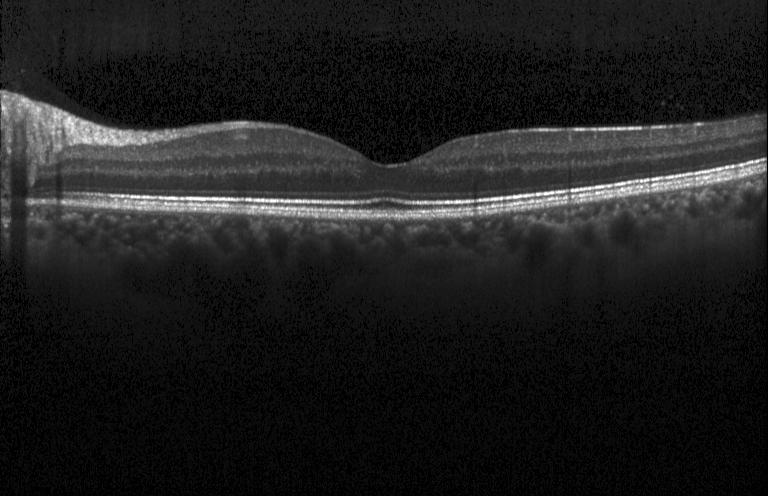 SD-OCT, OCT line scan. Diagnosis: no choroidal neovascularization, diabetic macular edema, or drusen.